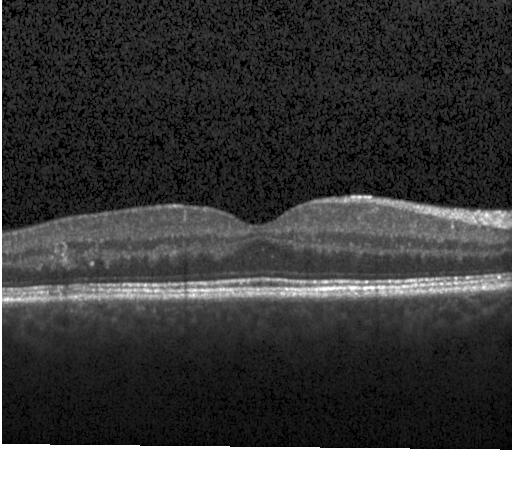
Instrument: Heidelberg Spectralis. Spectral-domain OCT. Centered on the fovea. Retinal OCT B-scan — Impression: no evidence of choroidal neovascularization, diabetic macular edema, or drusen.